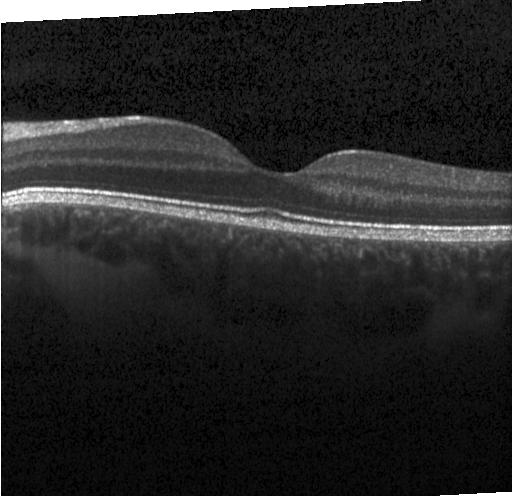

Macular OCT: neither choroidal neovascularization, diabetic macular edema, nor drusen.